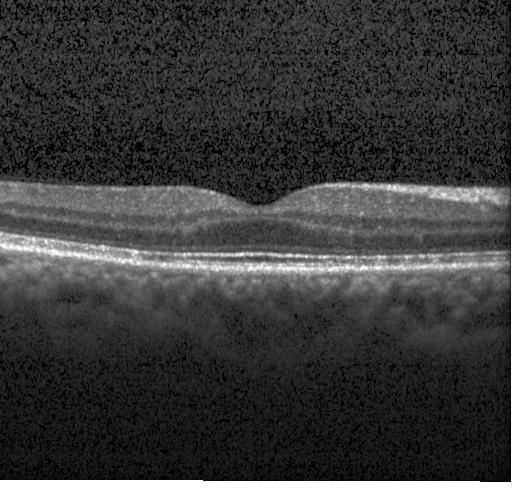
Spectral-domain OCT. Heidelberg Spectralis OCT system. Through the macula. OCT line scan — The scan shows no choroidal neovascularization, diabetic macular edema, or drusen.